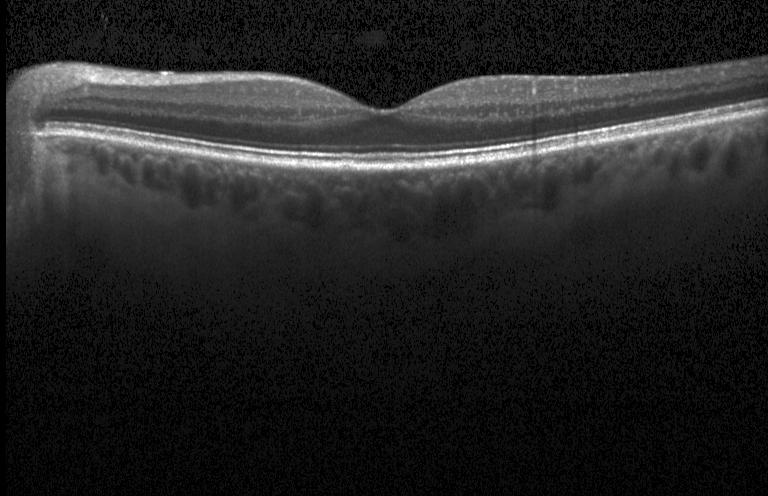 No choroidal neovascularization, no diabetic macular edema, and no drusen.